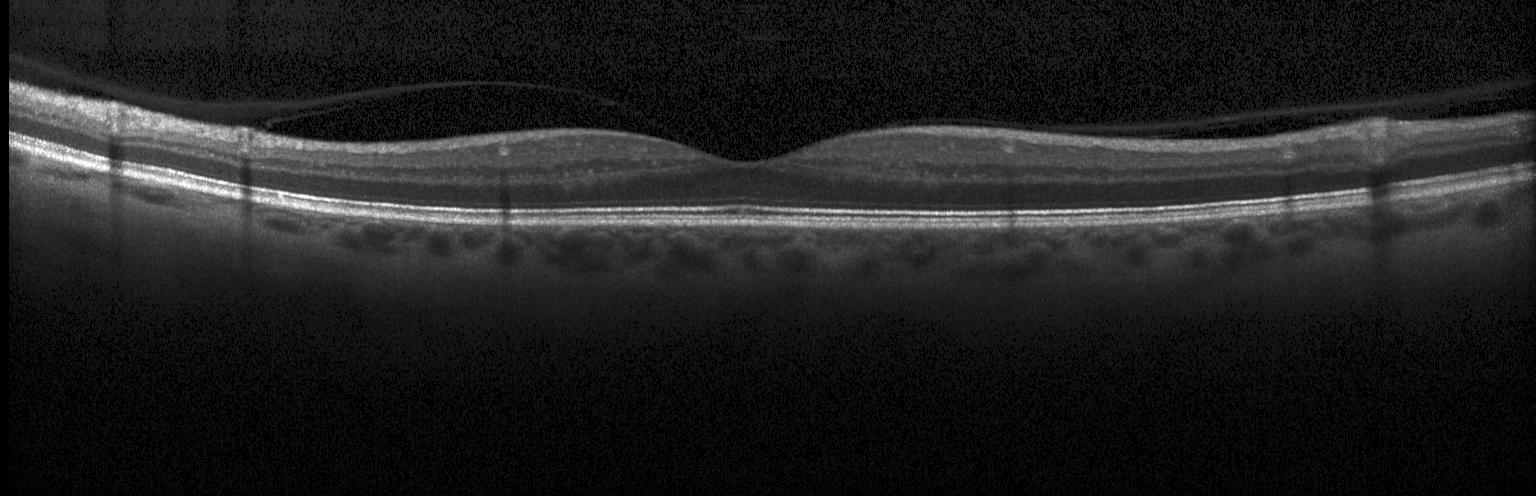 Impression: no evidence of choroidal neovascularization, diabetic macular edema, or drusen.